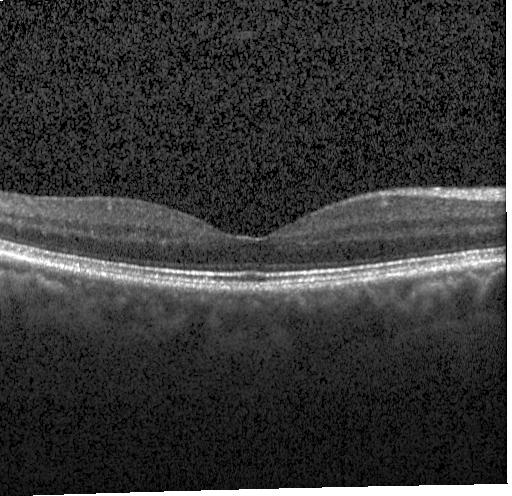

Optical coherence tomography B-scan.
Assessment: neither CNV, DME, nor drusen.